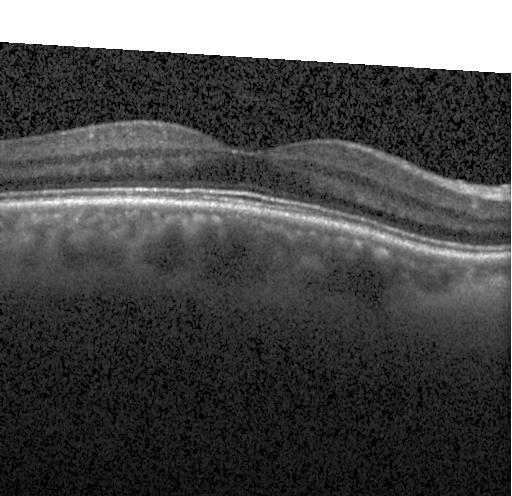

Retinal OCT cross-section, spectral-domain optical coherence tomography, instrument: Heidelberg Spectralis. Impression: neither CNV, DME, nor drusen.